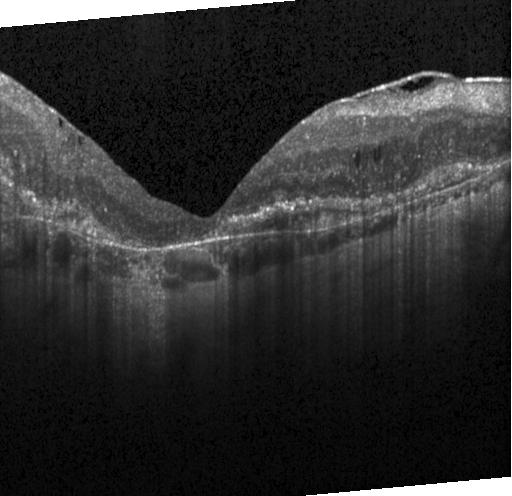

Spectral-domain OCT; Heidelberg Spectralis; horizontal scan through the fovea; optical coherence tomography scan.
Dx: a choroidal neovascular membrane.